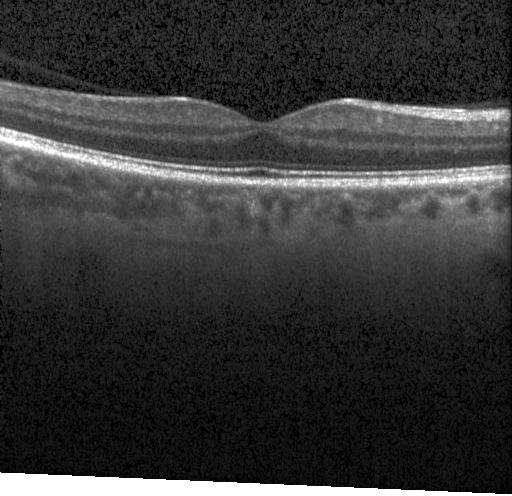 Diagnosis: no evidence of choroidal neovascularization, diabetic macular edema, or drusen.